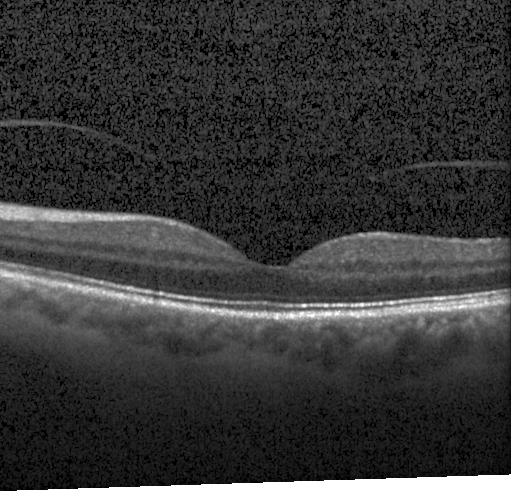
Spectral-domain OCT B-scan: no choroidal neovascularization, diabetic macular edema, or drusen.